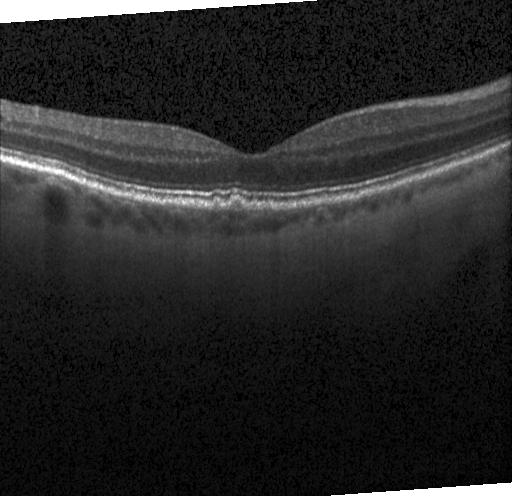
Centered on the fovea; Heidelberg Spectralis OCT system; optical coherence tomography scan
The scan shows multiple drusen.